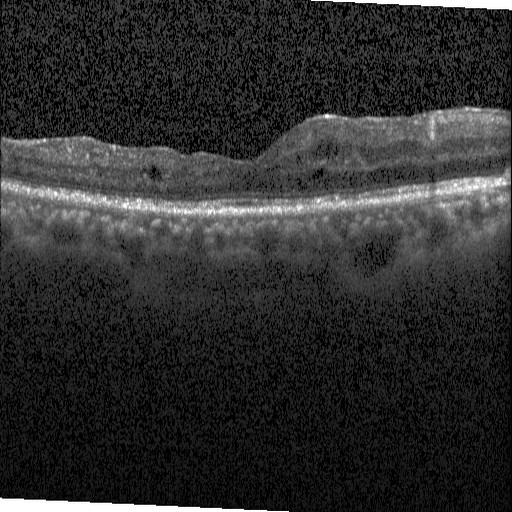

Heidelberg Spectralis, optical coherence tomography scan.
Impression: diabetic macular edema (DME).